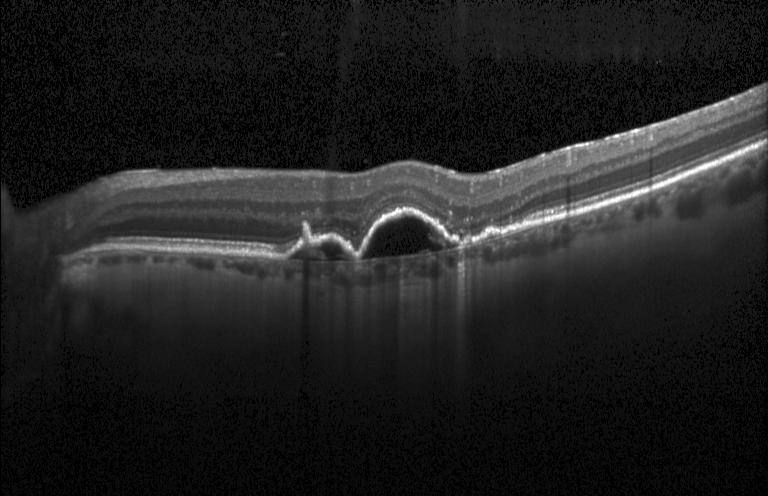 Heidelberg Spectralis OCT system. Retinal OCT B-scan. Spectral-domain optical coherence tomography.
Finding: choroidal neovascularization.